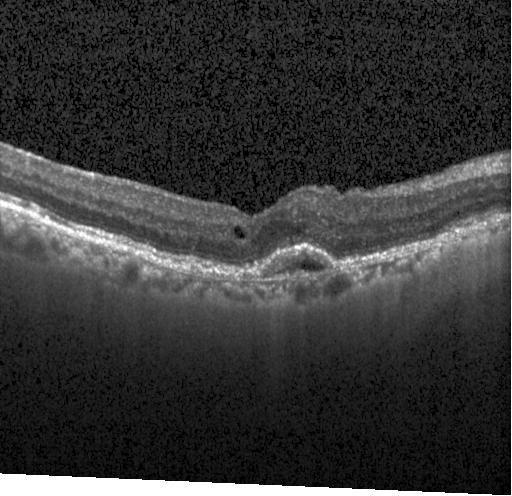

OCT B-scan showing choroidal neovascularization (CNV).